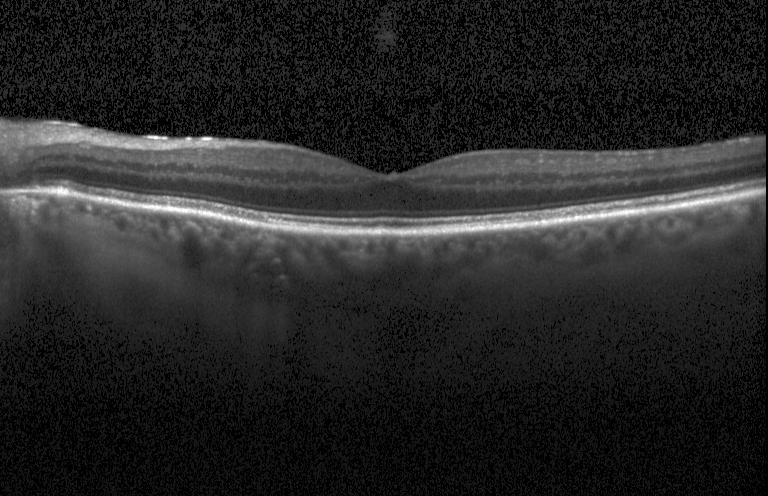

Diagnosis: no choroidal neovascularization, no diabetic macular edema, and no drusen.